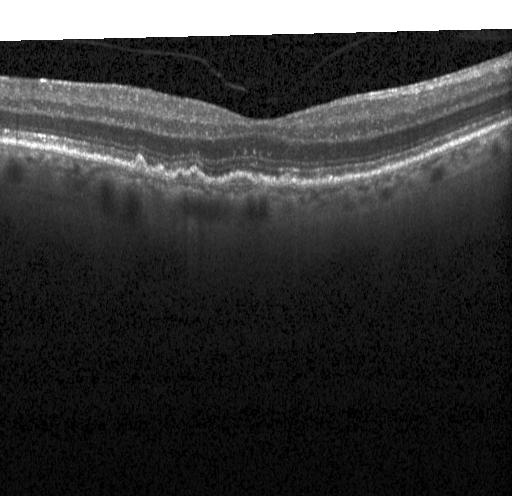

Impression: a choroidal neovascular membrane.